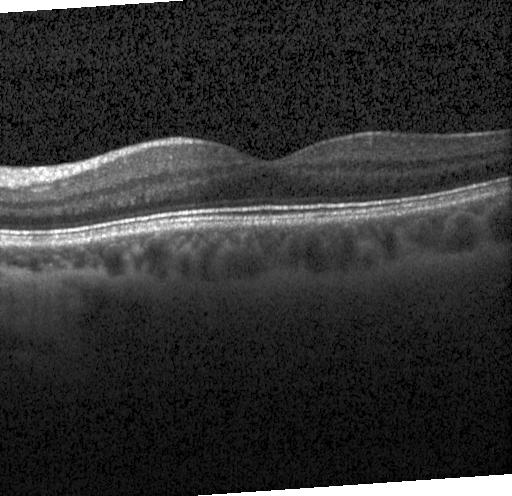

SD-OCT · retinal OCT B-scan.
Finding: no evidence of choroidal neovascularization, diabetic macular edema, or drusen.